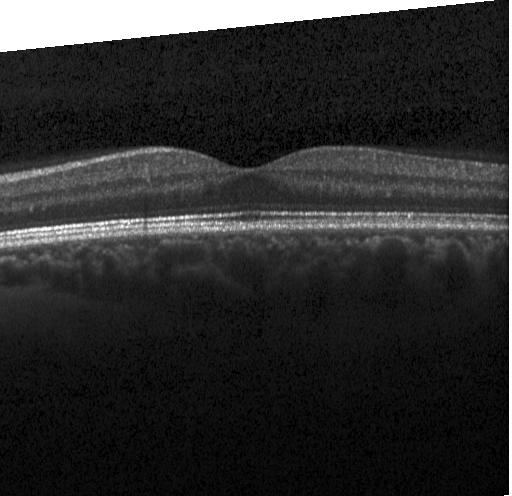
Diagnosis: no CNV, DME, or drusen.